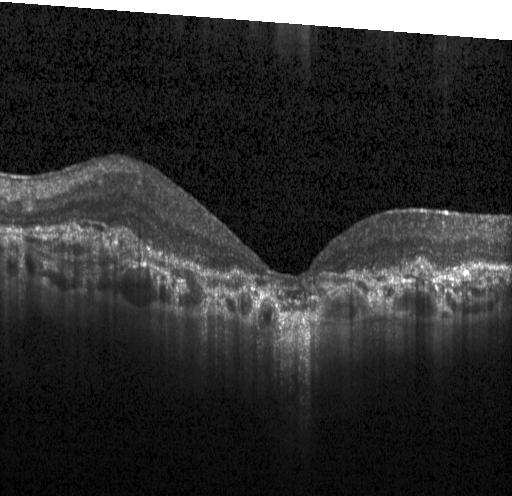 Retinal OCT cross-section showing CNV.